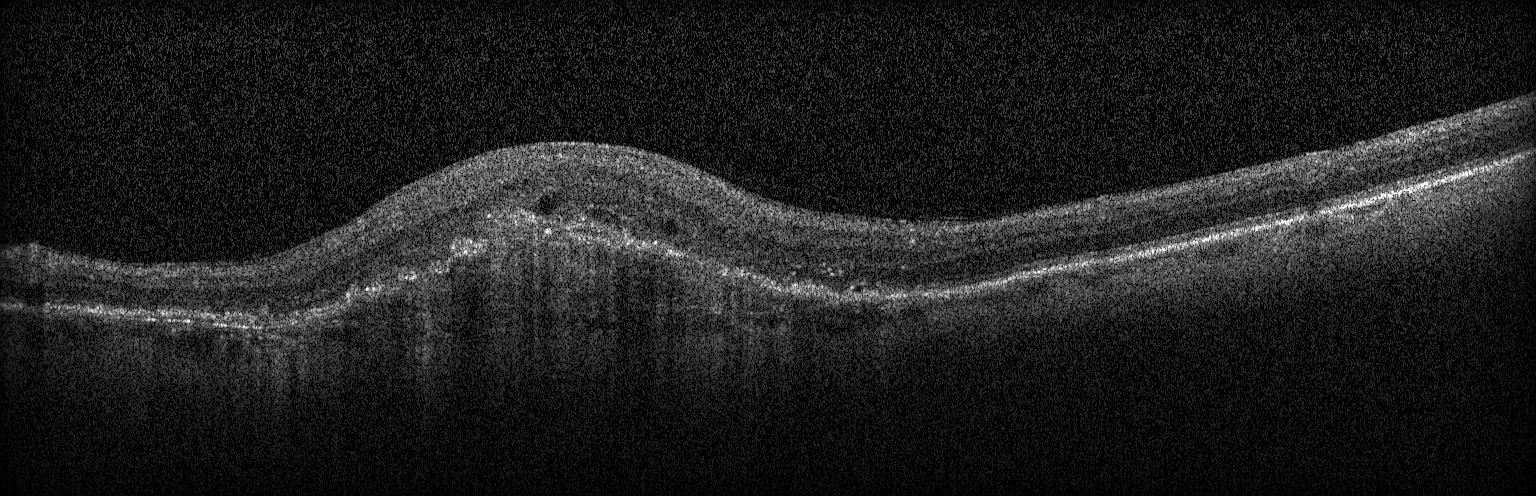
Diagnosis: choroidal neovascularization (CNV).